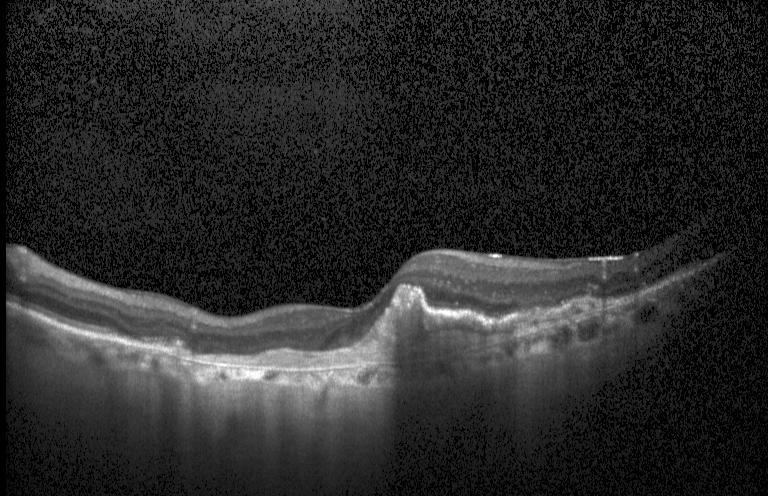

Retinal OCT B-scan, SD-OCT, instrument: Heidelberg Spectralis — Finding: choroidal neovascularization.